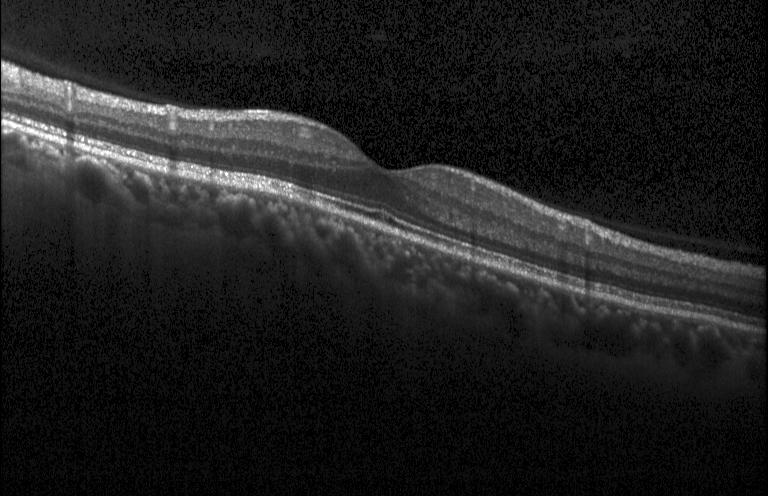 Spectral-domain optical coherence tomography; OCT B-scan — OCT finding: no choroidal neovascularization, no diabetic macular edema, and no drusen.